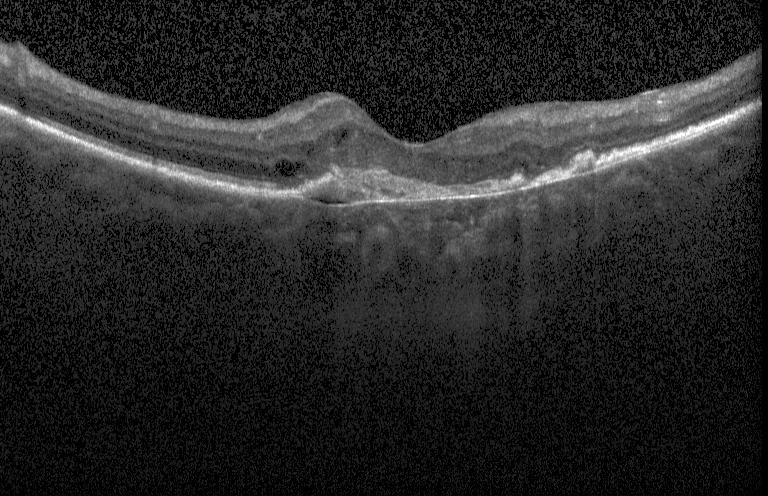 The scan shows CNV.